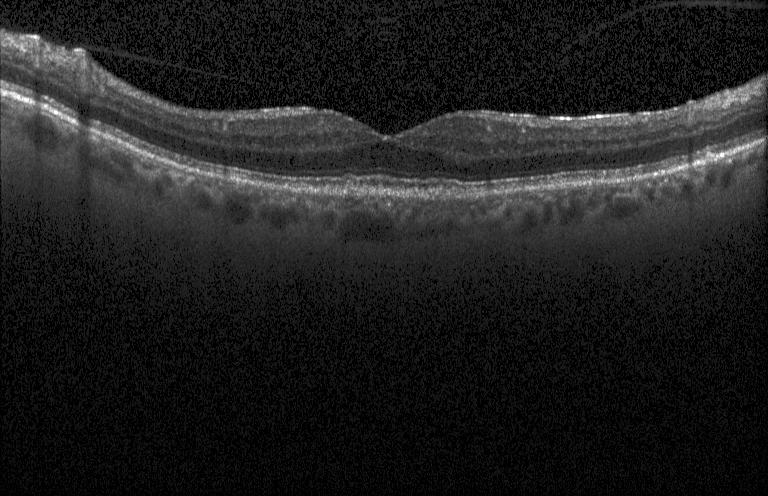
Optical coherence tomography B-scan, Heidelberg Spectralis OCT system, spectral-domain OCT, macular scan.
OCT finding: drusen.